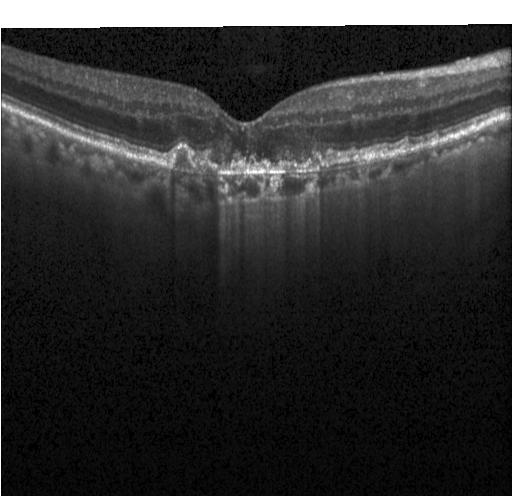
Spectral-domain OCT; acquired on a Heidelberg Spectralis; OCT line scan. The scan shows a choroidal neovascular membrane.